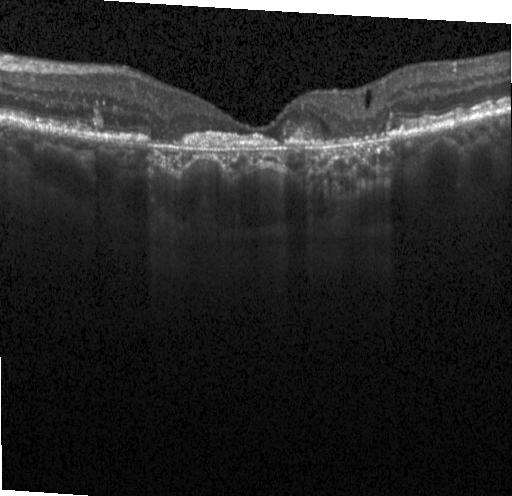
Instrument: Heidelberg Spectralis · SD-OCT · macular scan · retinal OCT B-scan
Impression: a choroidal neovascular membrane.